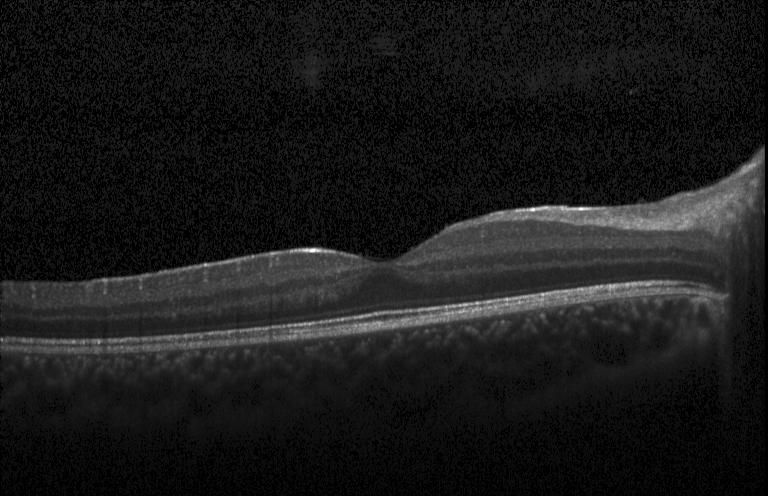

Optical coherence tomography scan.
The scan shows no choroidal neovascularization, diabetic macular edema, or drusen.